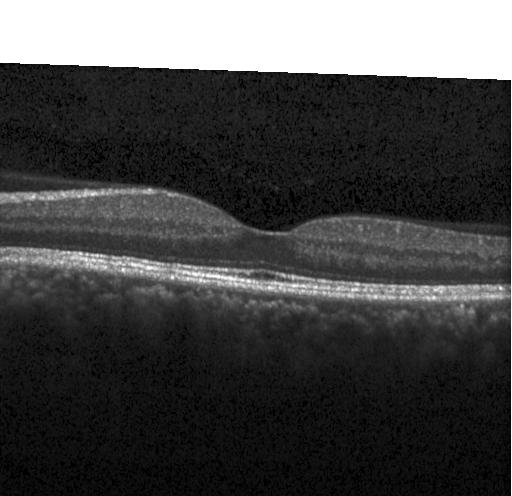

OCT B-scan.
Finding: no choroidal neovascularization, diabetic macular edema, or drusen.